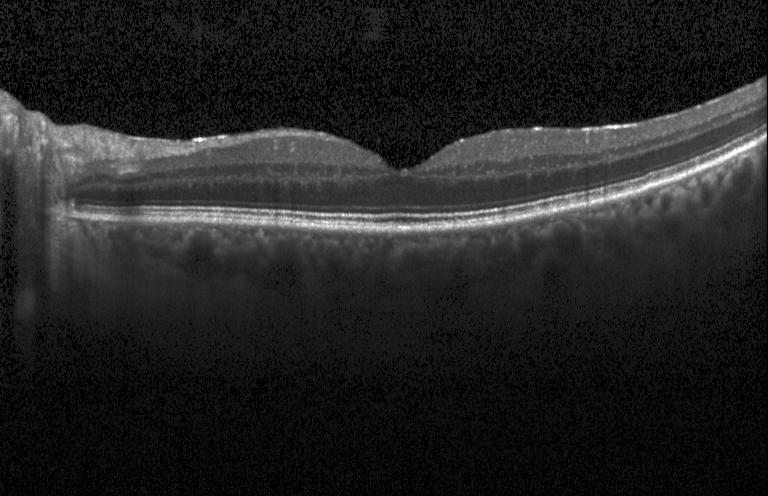
Dx: neither CNV, DME, nor drusen.